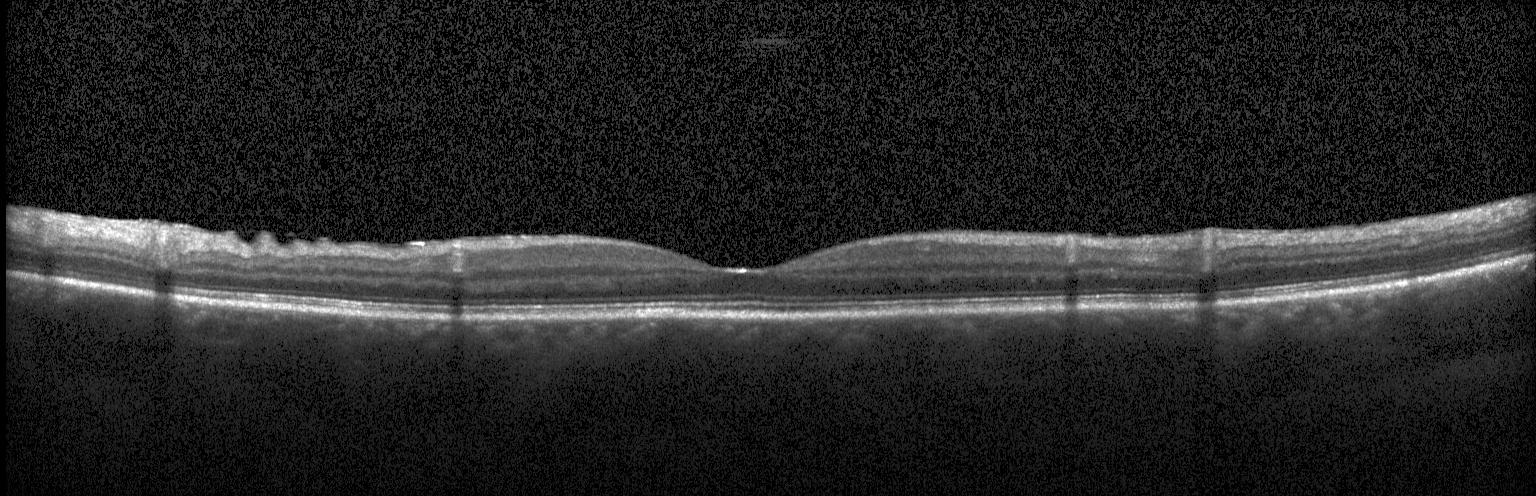
Impression: no evidence of choroidal neovascularization, diabetic macular edema, or drusen.